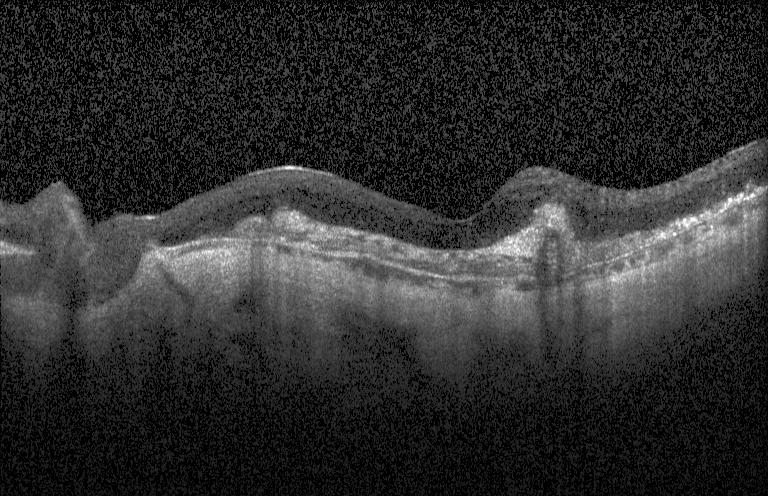
Fovea-centered. OCT B-scan. Acquired on a Heidelberg Spectralis.
Assessment: a choroidal neovascular membrane.